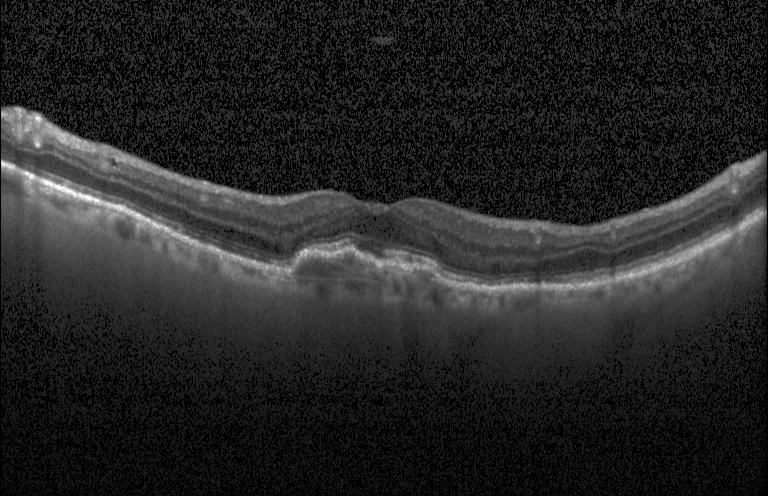 Retinal OCT cross-section — Finding: a choroidal neovascular membrane.